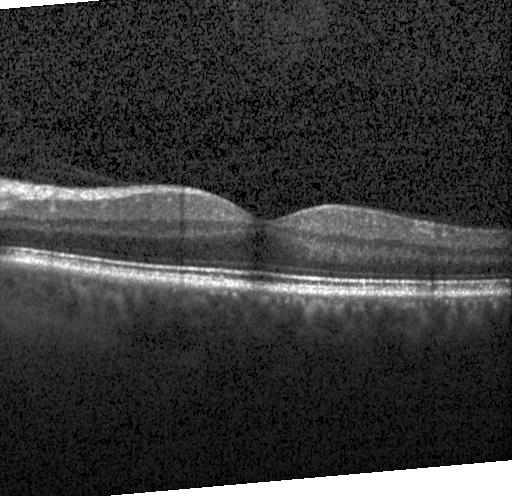

Diagnosis: no choroidal neovascularization, diabetic macular edema, or drusen.